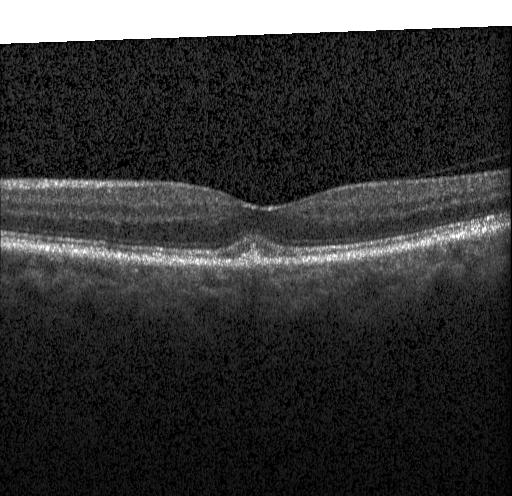

OCT line scan. Instrument: Heidelberg Spectralis
Dx: multiple drusen.